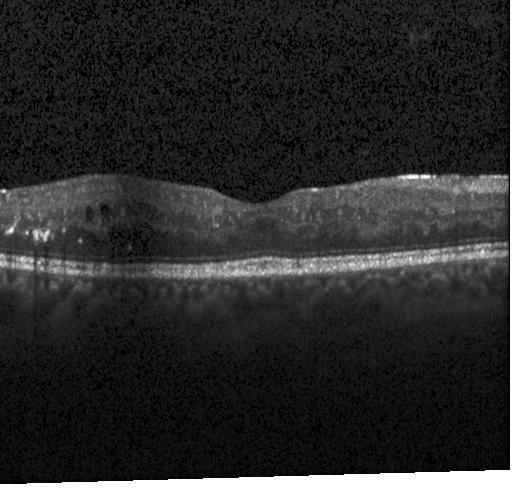
Impression: diabetic macular edema (DME).